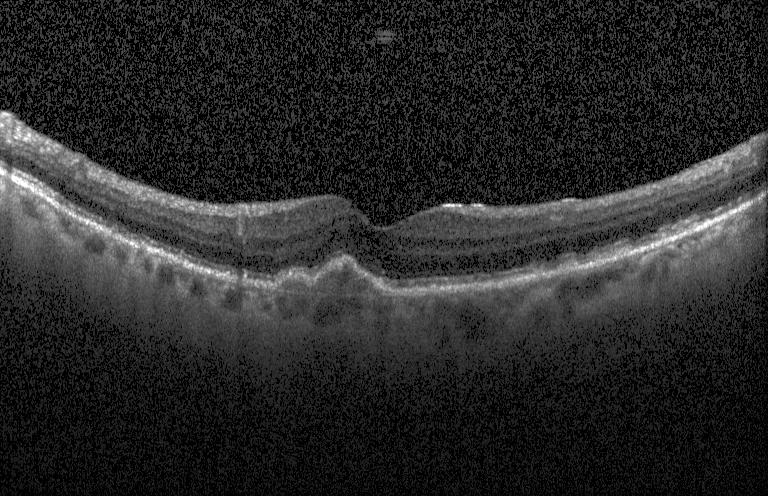
Retinal OCT B-scan, macular scan.
Diagnosis: a choroidal neovascular membrane.